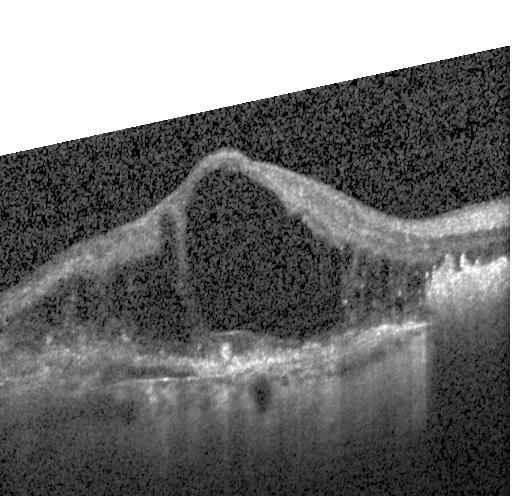
Optical coherence tomography B-scan, macular scan, SD-OCT
OCT finding: CNV.